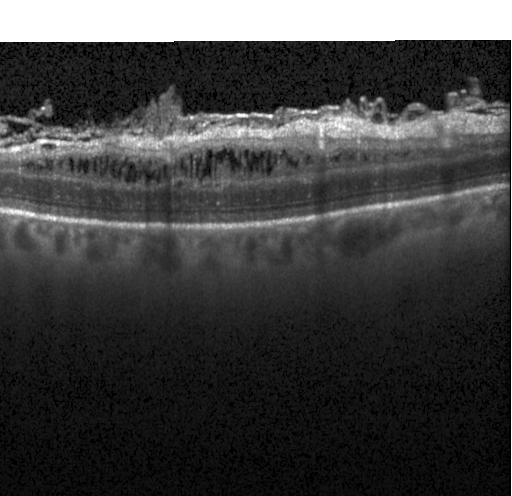 Heidelberg Spectralis OCT system; optical coherence tomography B-scan; macular scan — Macular OCT: DME.